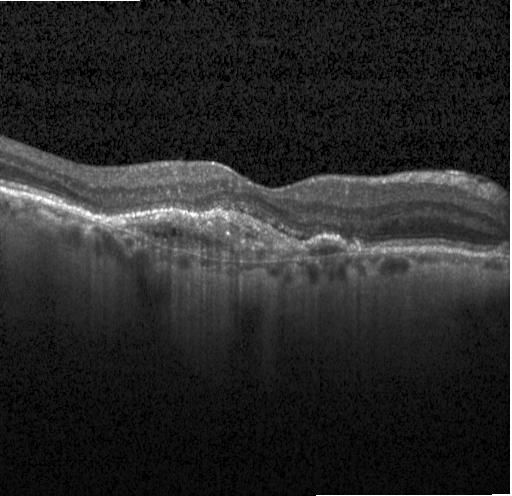
Horizontal scan through the fovea · retinal OCT B-scan · spectral-domain OCT · acquired on a Heidelberg Spectralis.
This B-scan demonstrates choroidal neovascularization.